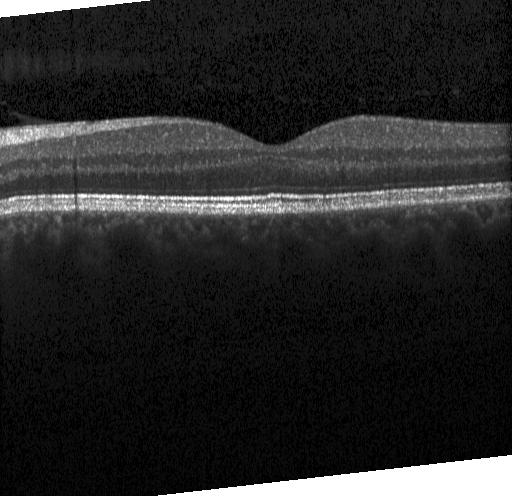 OCT line scan; horizontal scan through the fovea.
This B-scan demonstrates neither choroidal neovascularization, diabetic macular edema, nor drusen.